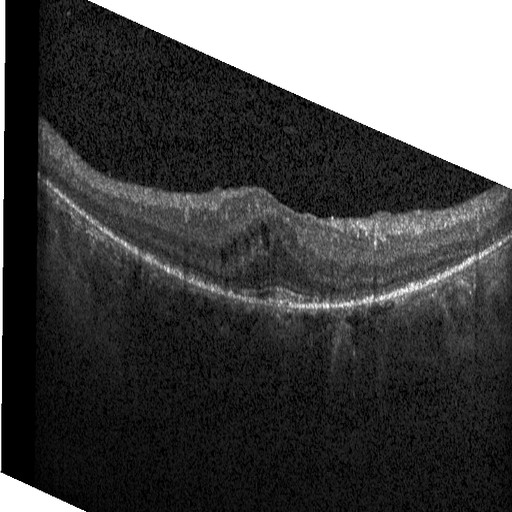 OCT line scan — This B-scan demonstrates diabetic macular edema (DME).